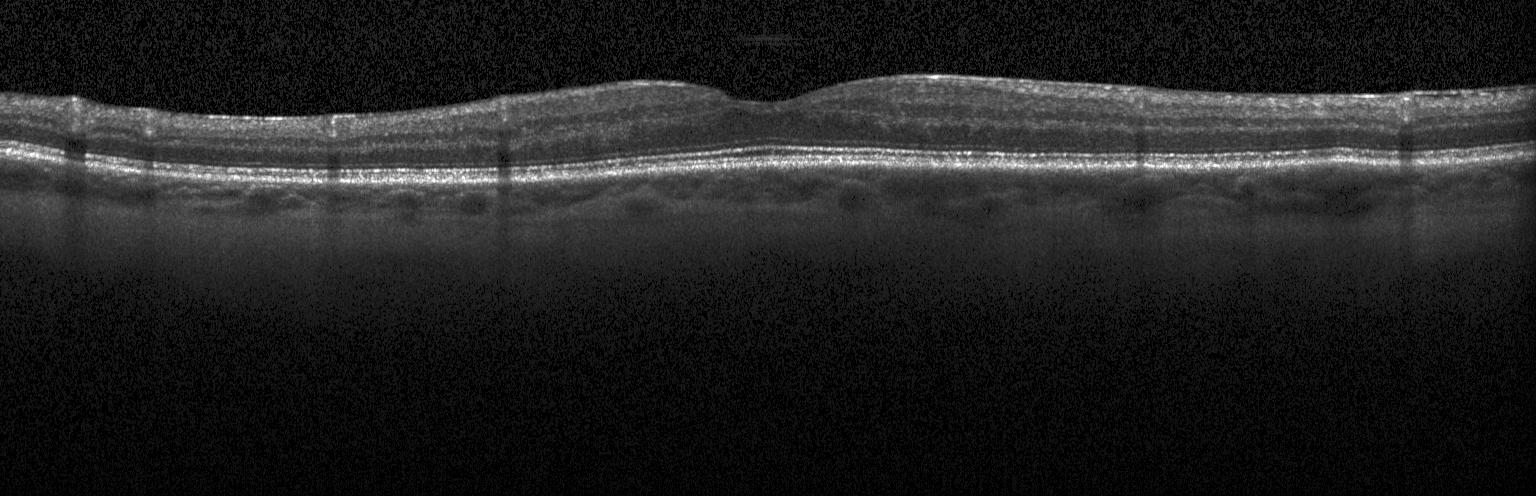

Optical coherence tomography scan. Heidelberg Spectralis OCT system. Spectral-domain OCT. Macular OCT: no choroidal neovascularization, diabetic macular edema, or drusen.